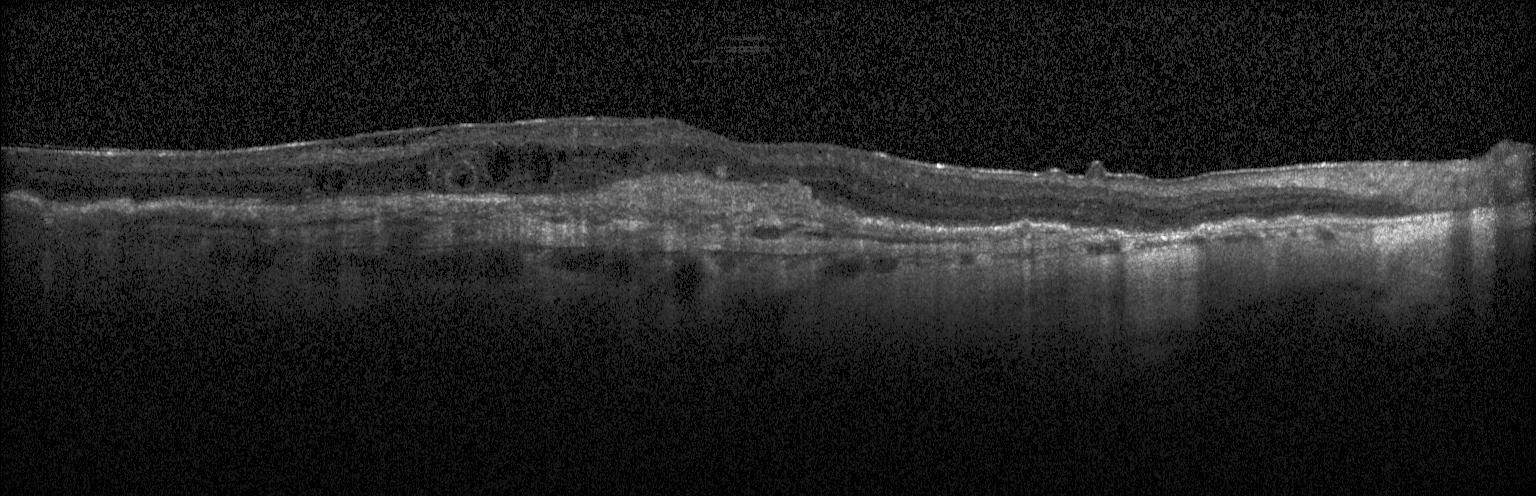
Dx: choroidal neovascularization (CNV).